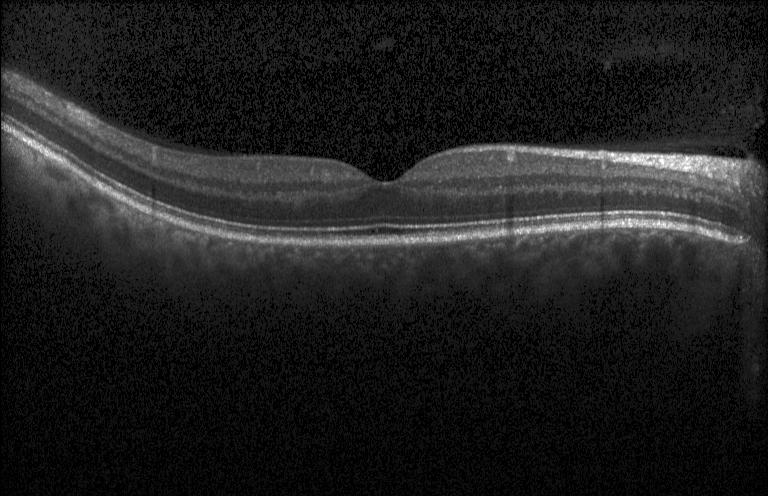 OCT finding: neither choroidal neovascularization, diabetic macular edema, nor drusen.